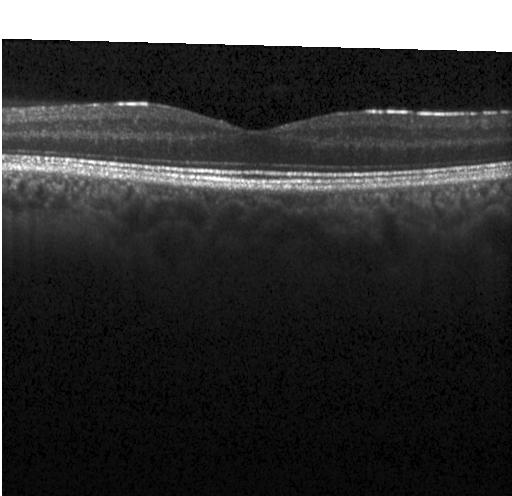

Heidelberg Spectralis. Spectral-domain OCT. Retinal OCT cross-section. Macular scan
Impression: no choroidal neovascularization, diabetic macular edema, or drusen.